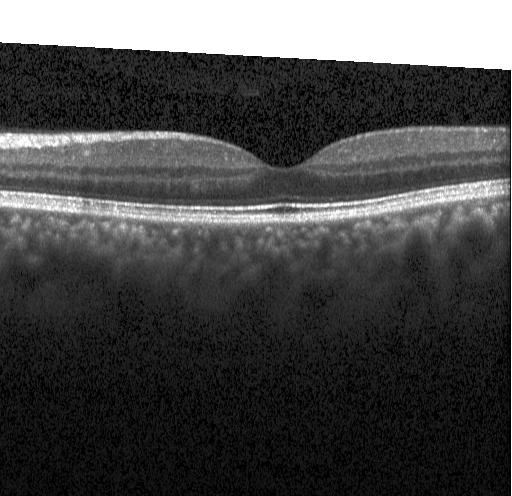
OCT B-scan showing no choroidal neovascularization, no diabetic macular edema, and no drusen.